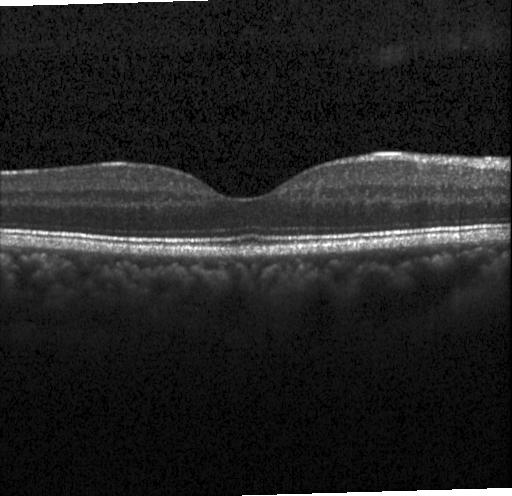
Macular OCT: no evidence of choroidal neovascularization, diabetic macular edema, or drusen.